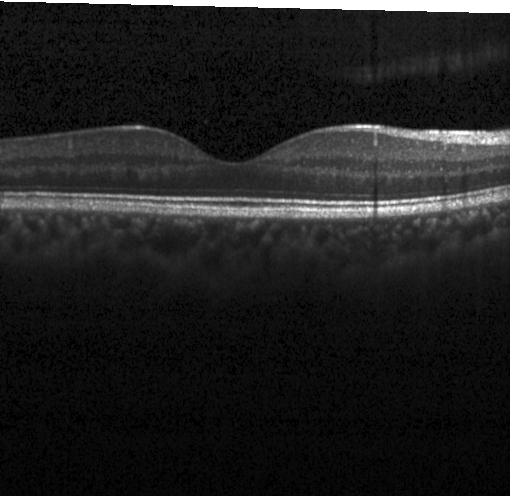 Optical coherence tomography B-scan — This B-scan demonstrates neither CNV, DME, nor drusen.